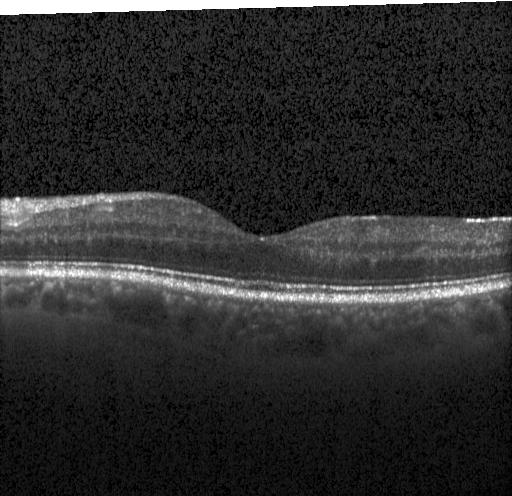 OCT B-scan
Diagnosis: neither choroidal neovascularization, diabetic macular edema, nor drusen.